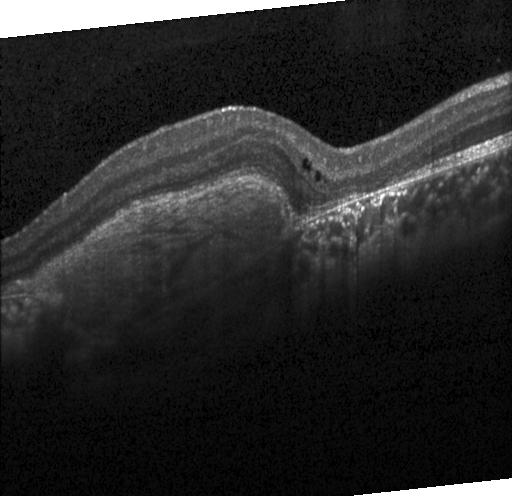 Optical coherence tomography B-scan. Instrument: Heidelberg Spectralis. Spectral-domain OCT.
Assessment: choroidal neovascularization (CNV).